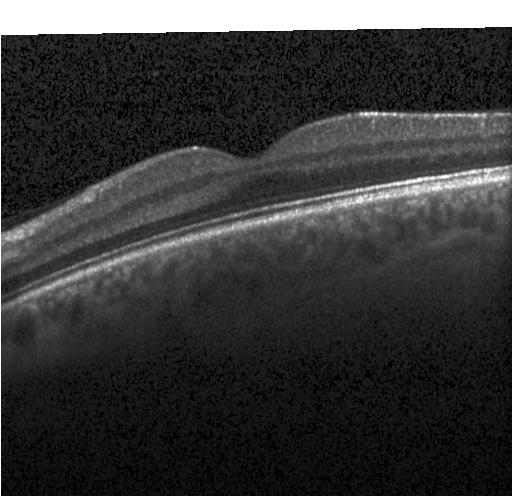
Finding: no CNV, DME, or drusen.